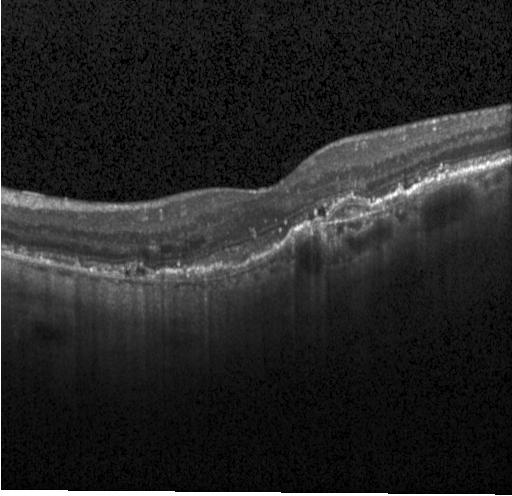 Impression: choroidal neovascularization (CNV).